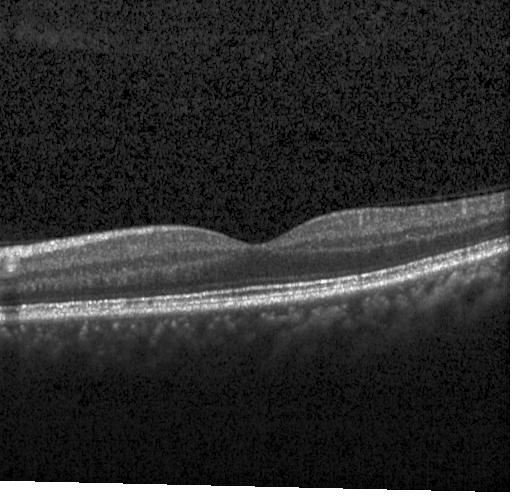
OCT B-scan. Impression: no evidence of choroidal neovascularization, diabetic macular edema, or drusen.